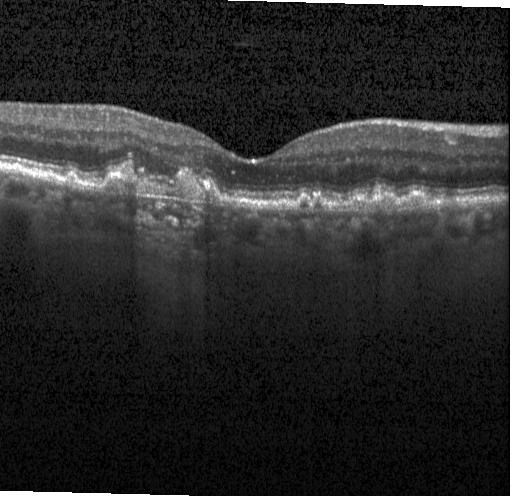

The scan shows choroidal neovascularization (CNV).